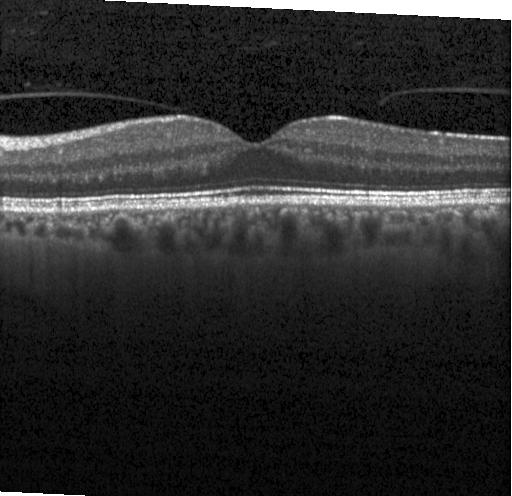

Centered on the fovea. Spectral-domain optical coherence tomography. Acquired on a Heidelberg Spectralis. OCT line scan. Macular OCT: no choroidal neovascularization, no diabetic macular edema, and no drusen.